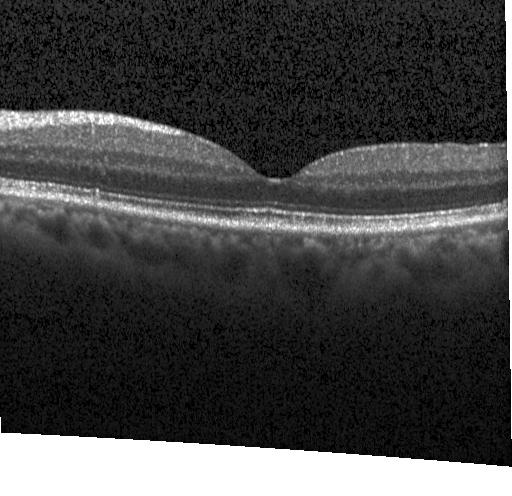
OCT B-scan, macular scan, spectral-domain OCT, acquired on a Heidelberg Spectralis.
OCT finding: no CNV, no DME, and no drusen.